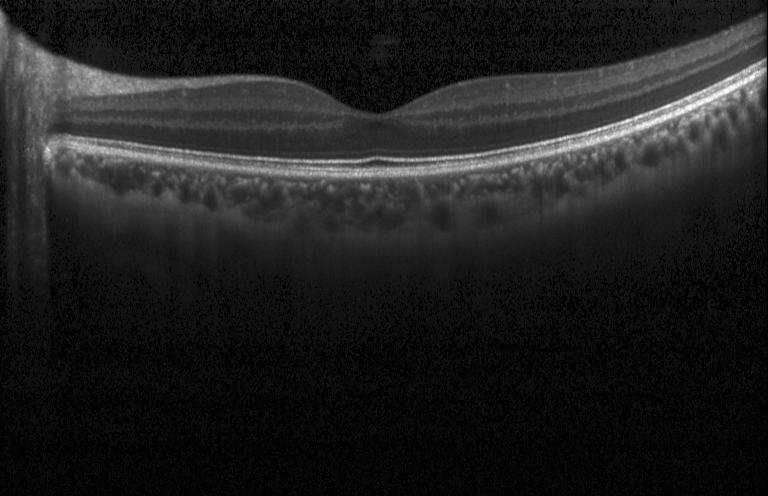 This B-scan demonstrates no choroidal neovascularization, diabetic macular edema, or drusen.